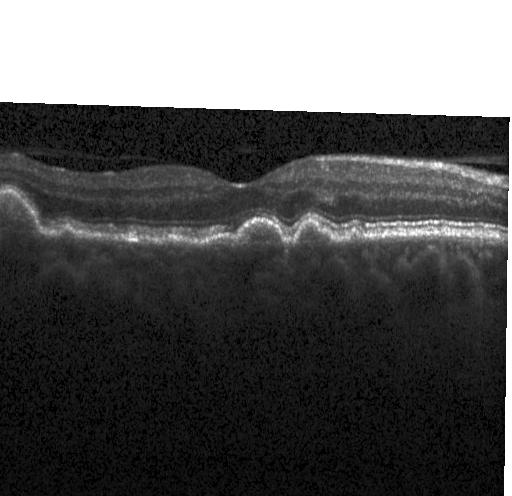

Optical coherence tomography scan; spectral-domain optical coherence tomography — Dx: drusen.